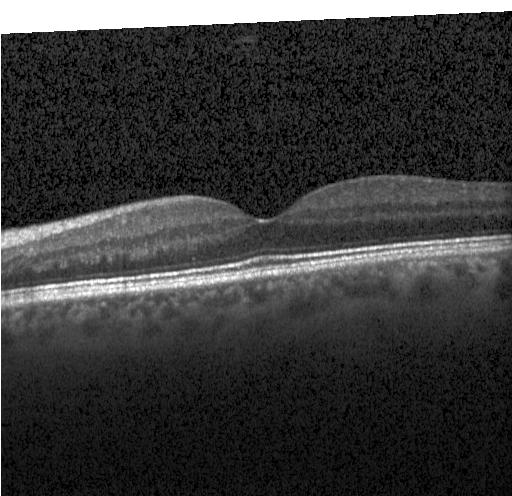

Impression: no choroidal neovascularization, diabetic macular edema, or drusen.